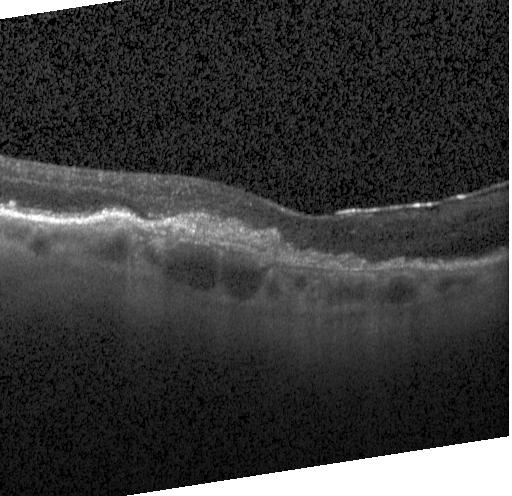
Macular OCT demonstrating CNV.